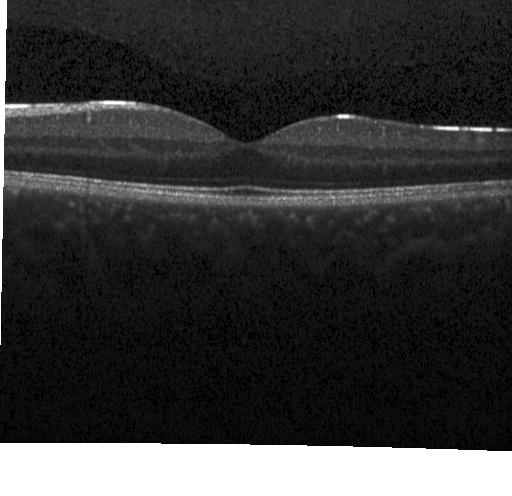

Finding: no choroidal neovascularization, diabetic macular edema, or drusen.